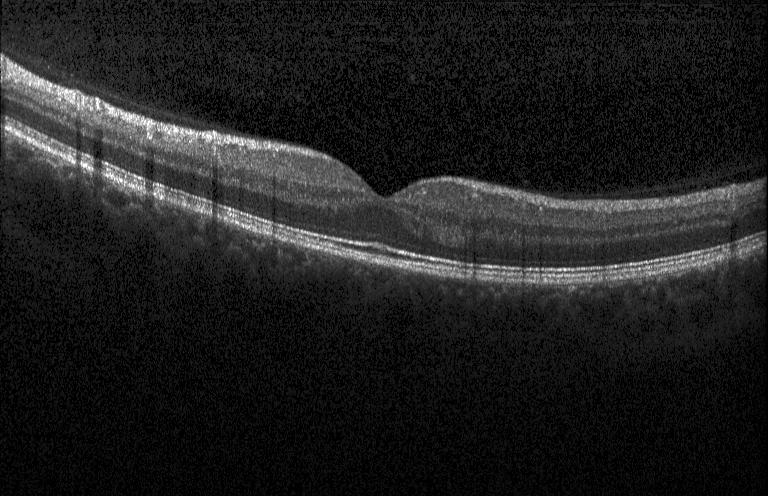 OCT finding: no evidence of choroidal neovascularization, diabetic macular edema, or drusen.